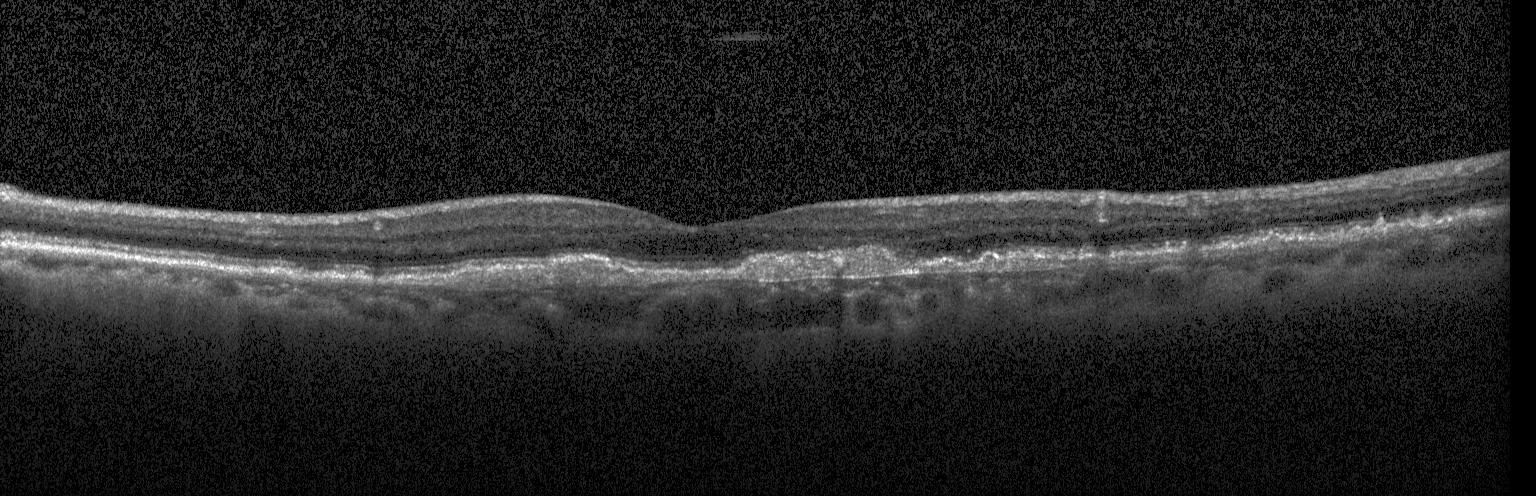 Diagnosis: a choroidal neovascular membrane.